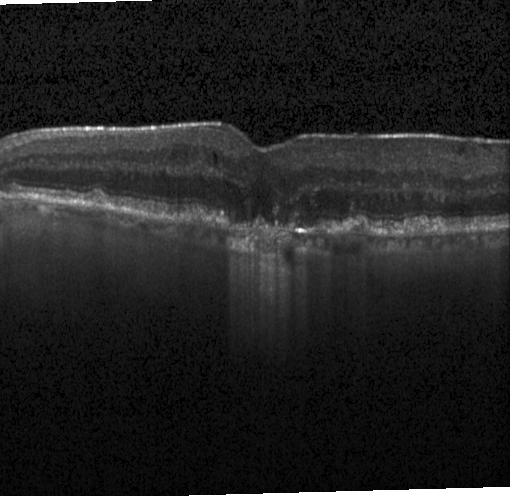
Optical coherence tomography B-scan; horizontal scan through the fovea — Assessment: CNV.